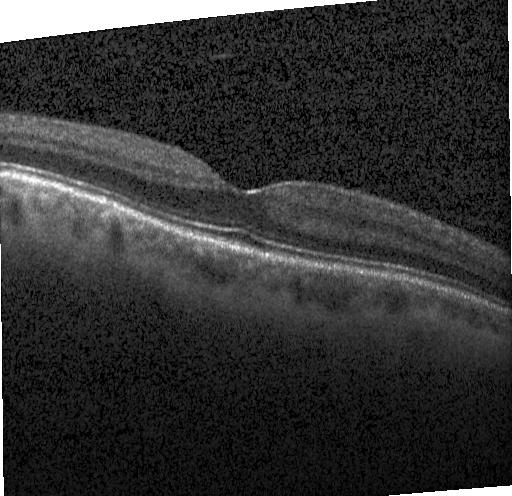
OCT B-scan, spectral-domain optical coherence tomography.
Assessment: neither choroidal neovascularization, diabetic macular edema, nor drusen.